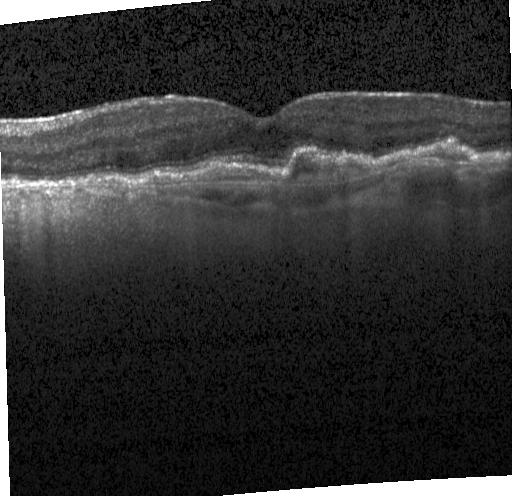
Impression: a choroidal neovascular membrane.